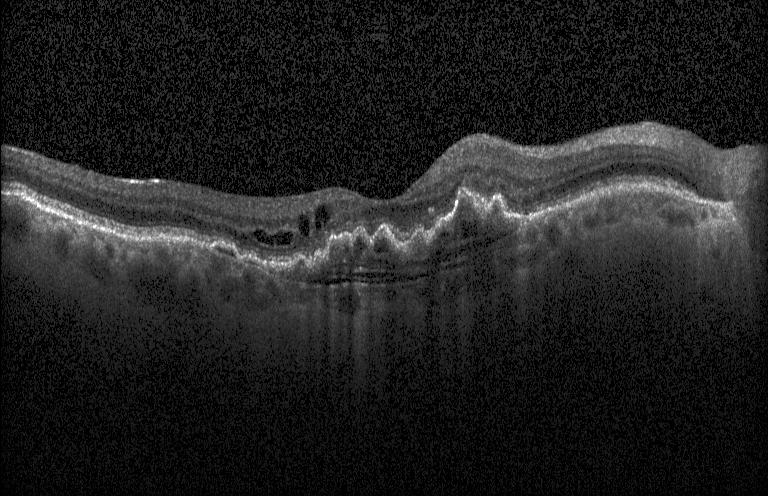

OCT finding: choroidal neovascularization.